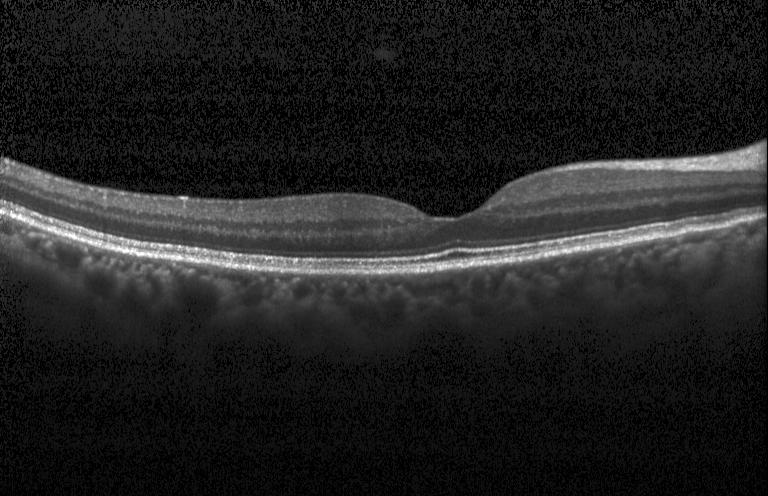 Spectral-domain OCT B-scan: neither choroidal neovascularization, diabetic macular edema, nor drusen.